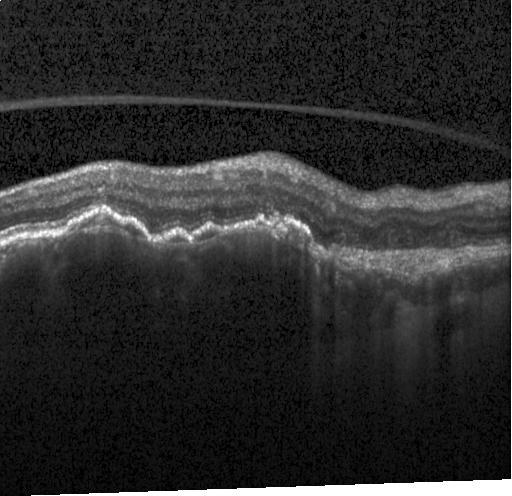 Diagnosis: a choroidal neovascular membrane.